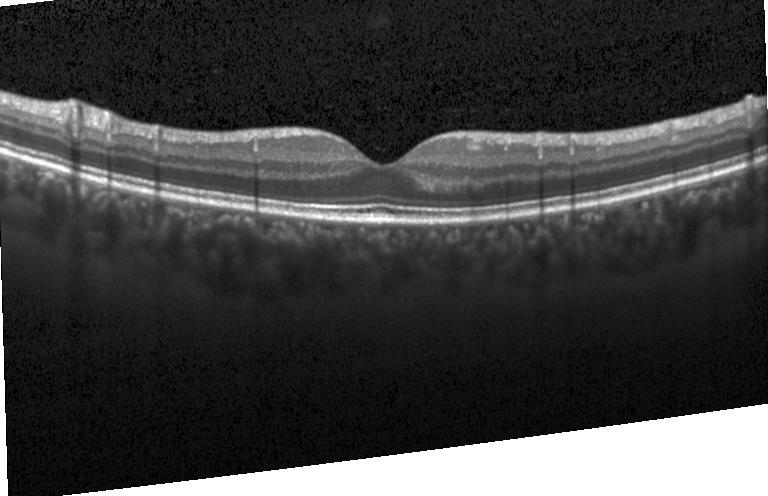 Retinal OCT cross-section
No choroidal neovascularization, no diabetic macular edema, and no drusen.